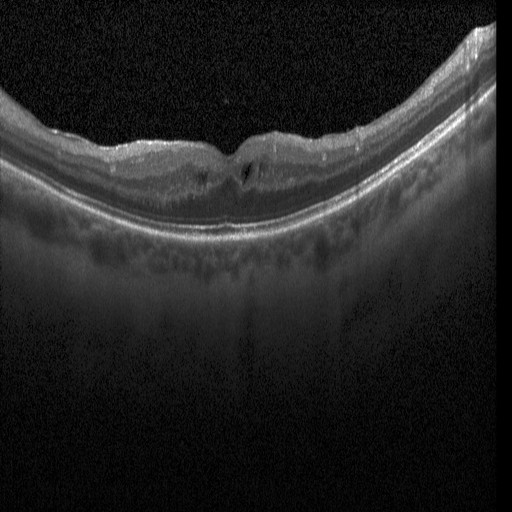
OCT B-scan — Diagnosis: DME.